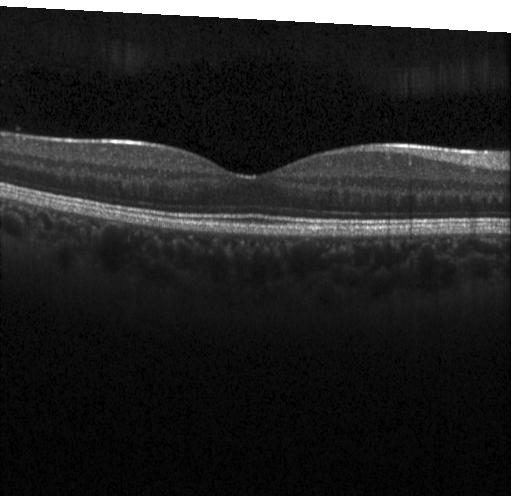
OCT line scan, Heidelberg Spectralis. Finding: no choroidal neovascularization, no diabetic macular edema, and no drusen.